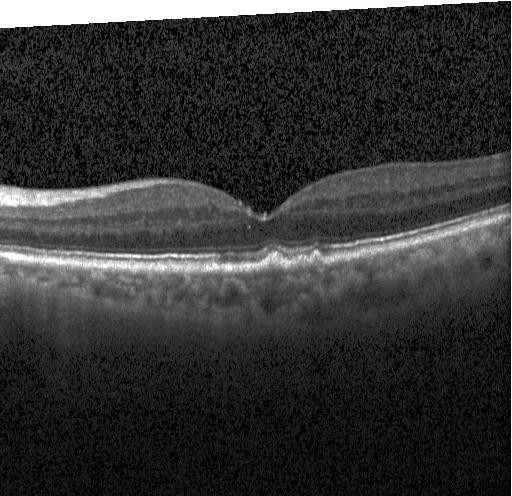 Diagnosis: drusen.